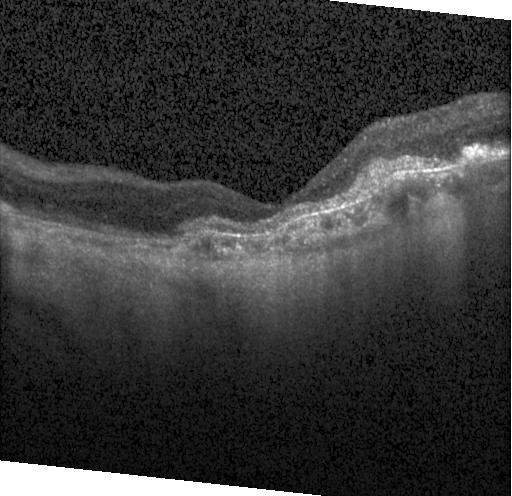
Macular scan · OCT B-scan · acquired on a Heidelberg Spectralis · spectral-domain optical coherence tomography.
A choroidal neovascular membrane.